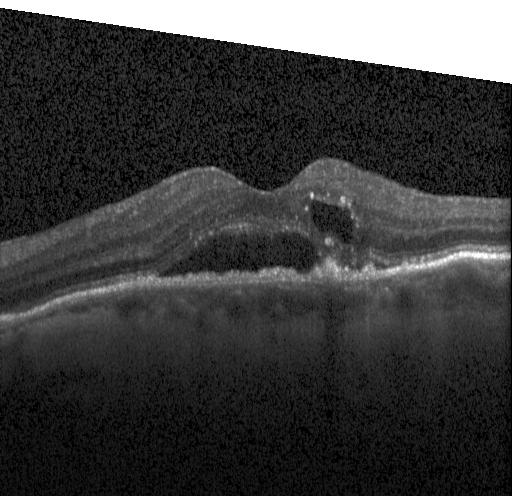 OCT B-scan. Horizontal scan through the fovea. Spectral-domain OCT.
Diagnosis: a choroidal neovascular membrane.